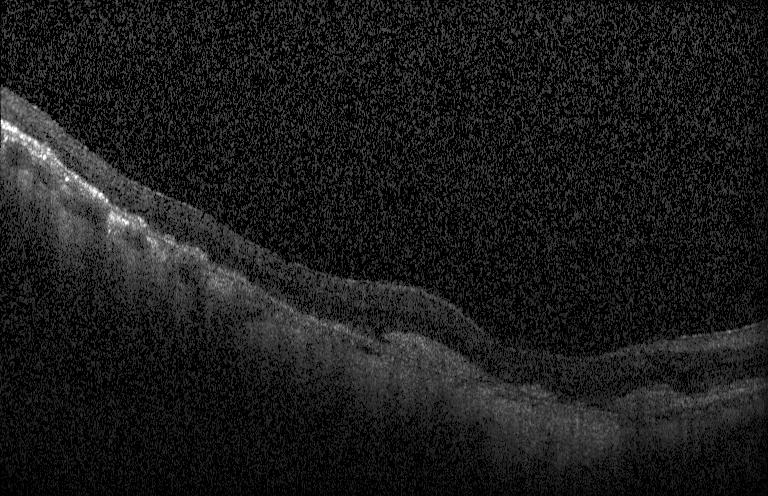

Macular OCT: choroidal neovascularization (CNV).